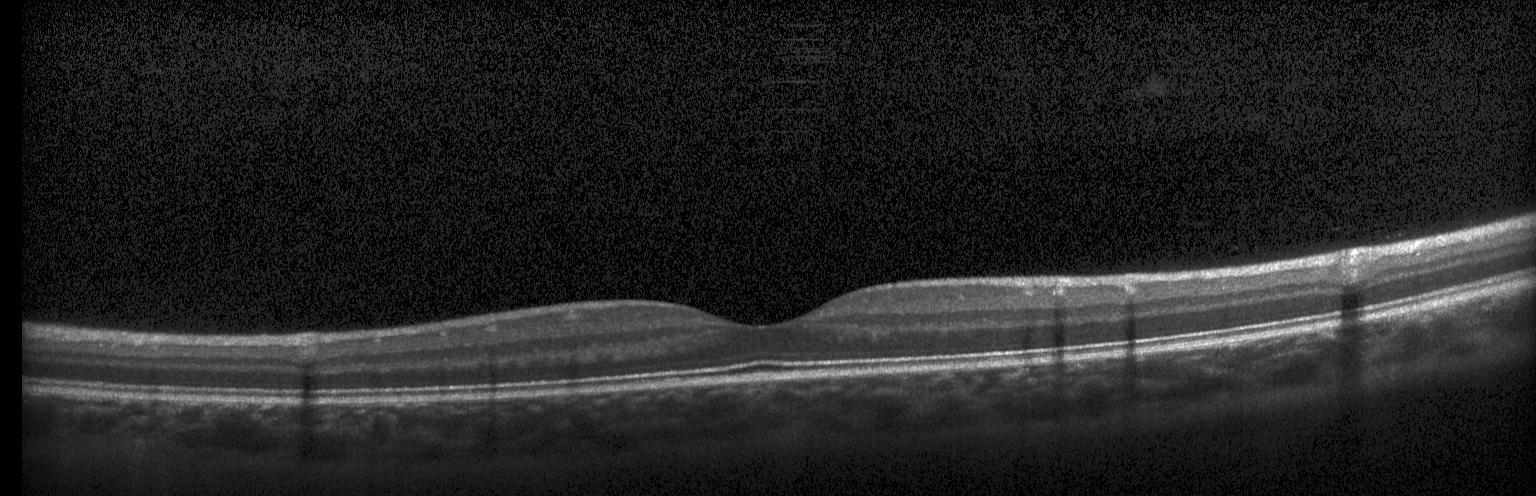

Macular OCT: neither CNV, DME, nor drusen.